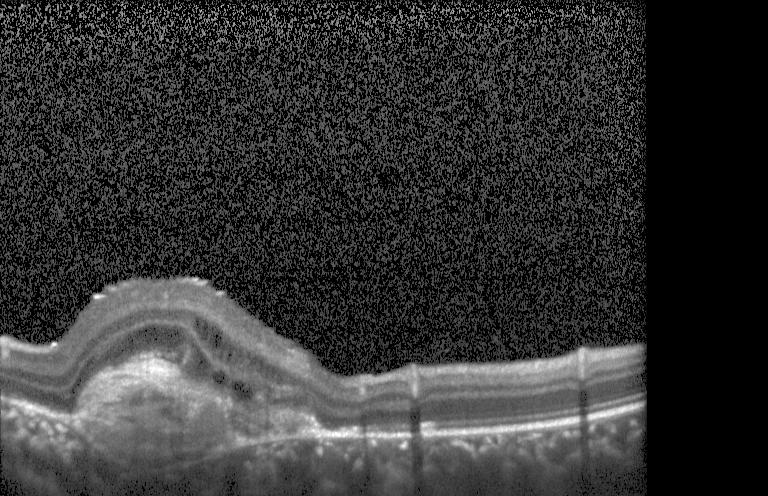

Retinal OCT B-scan — Macular OCT: a choroidal neovascular membrane.